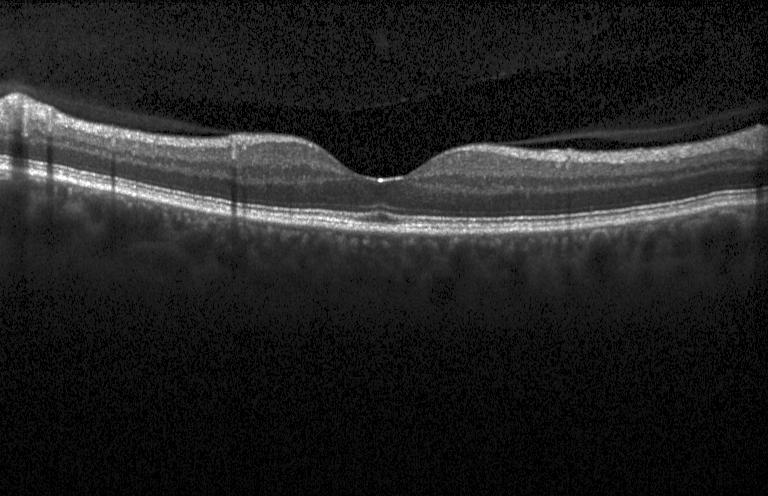
Spectral-domain optical coherence tomography. Fovea-centered. OCT line scan. Instrument: Heidelberg Spectralis
Diagnosis: no choroidal neovascularization, diabetic macular edema, or drusen.